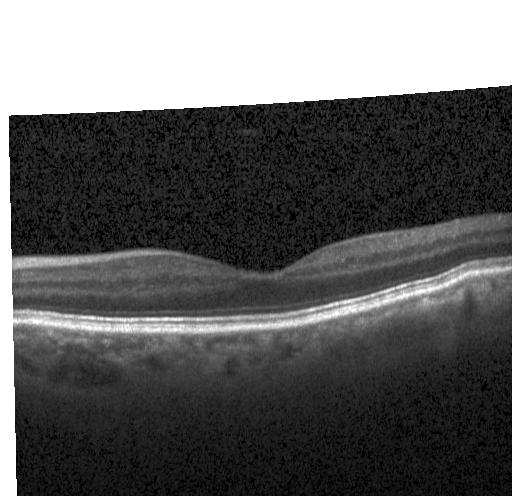
Optical coherence tomography scan. Spectral-domain optical coherence tomography. Acquired on a Heidelberg Spectralis. Centered on the fovea.
Dx: no choroidal neovascularization, diabetic macular edema, or drusen.